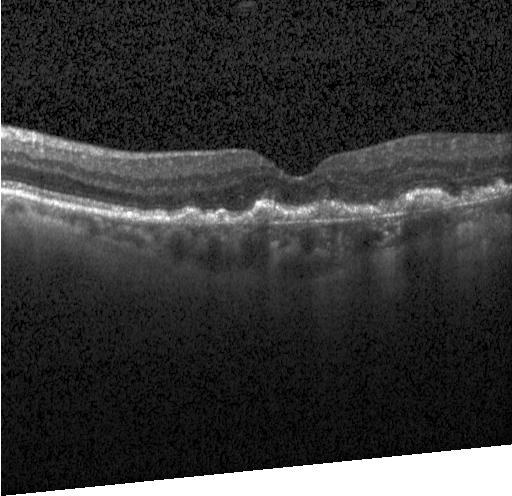
Retinal OCT cross-section showing choroidal neovascularization.